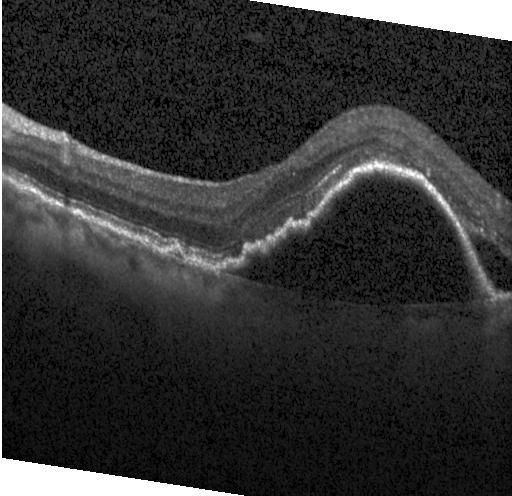
Optical coherence tomography scan — Impression: CNV.